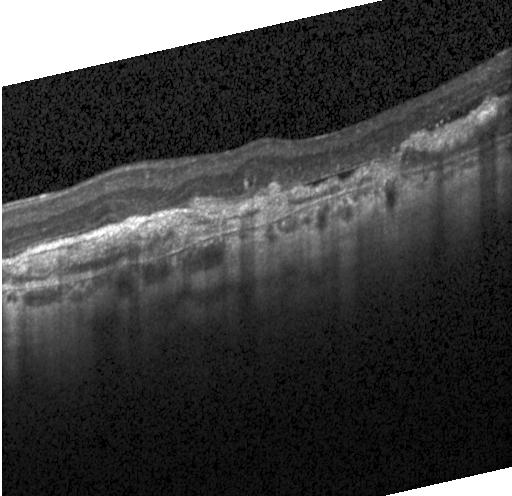
OCT B-scan · instrument: Heidelberg Spectralis · fovea-centered · spectral-domain optical coherence tomography
OCT finding: a choroidal neovascular membrane.